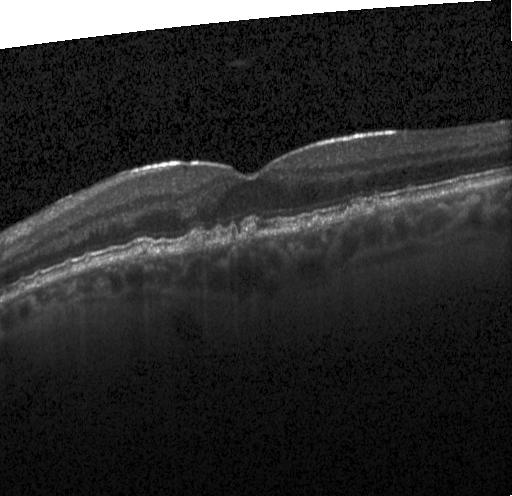

OCT finding: multiple drusen.